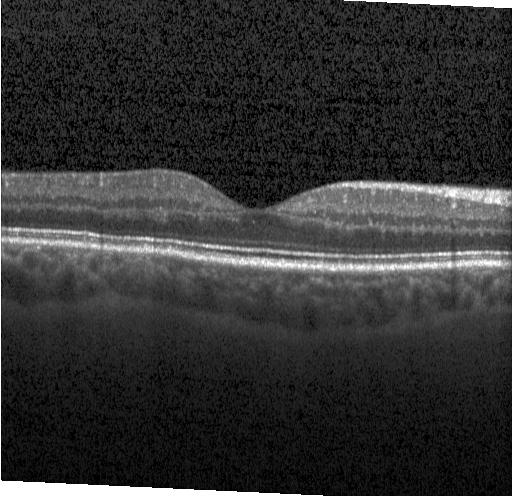 Instrument: Heidelberg Spectralis, optical coherence tomography scan — Assessment: no evidence of choroidal neovascularization, diabetic macular edema, or drusen.